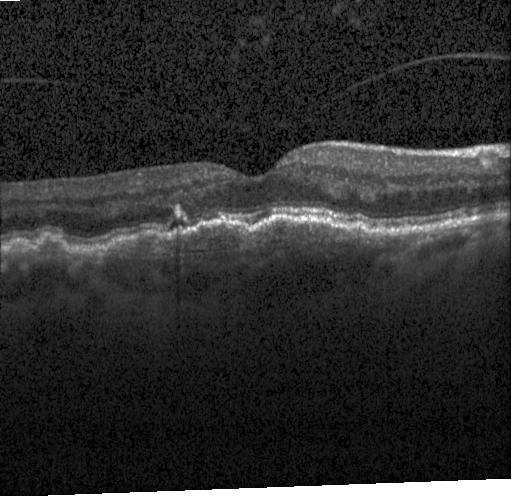 Diagnosis: a choroidal neovascular membrane.